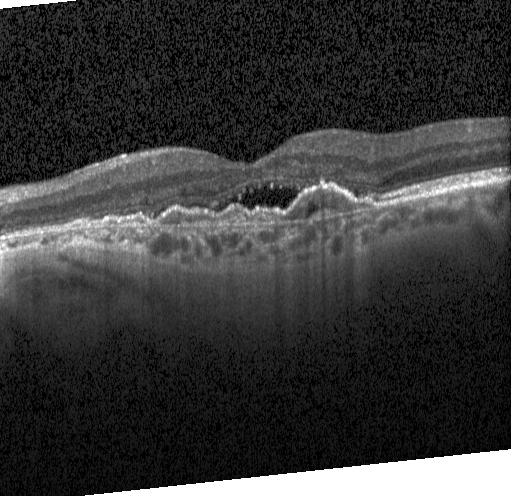
Heidelberg Spectralis OCT system; horizontal scan through the fovea; OCT B-scan; spectral-domain optical coherence tomography
This B-scan demonstrates choroidal neovascularization (CNV).